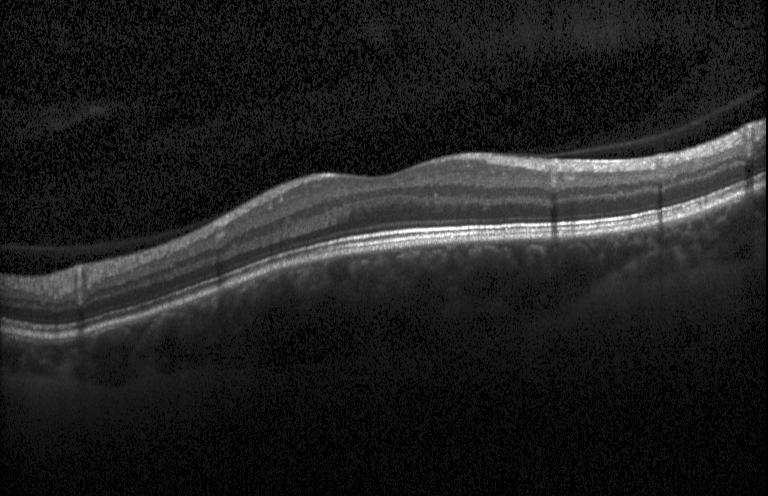
Acquired on a Heidelberg Spectralis; fovea-centered; retinal OCT cross-section; spectral-domain optical coherence tomography — Diagnosis: no evidence of choroidal neovascularization, diabetic macular edema, or drusen.